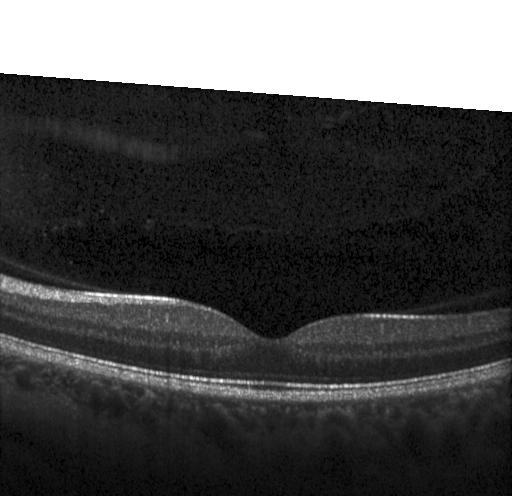 Horizontal scan through the fovea · optical coherence tomography scan · Heidelberg Spectralis OCT system.
Impression: neither choroidal neovascularization, diabetic macular edema, nor drusen.